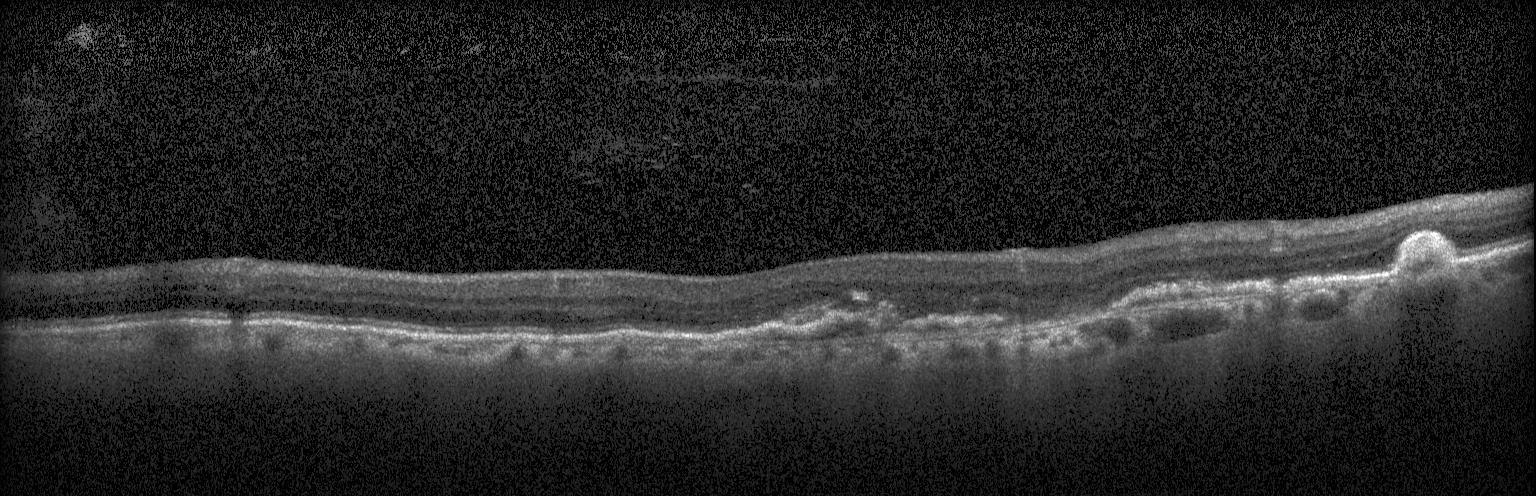

Through the macula, OCT B-scan, spectral-domain OCT.
Assessment: a choroidal neovascular membrane.